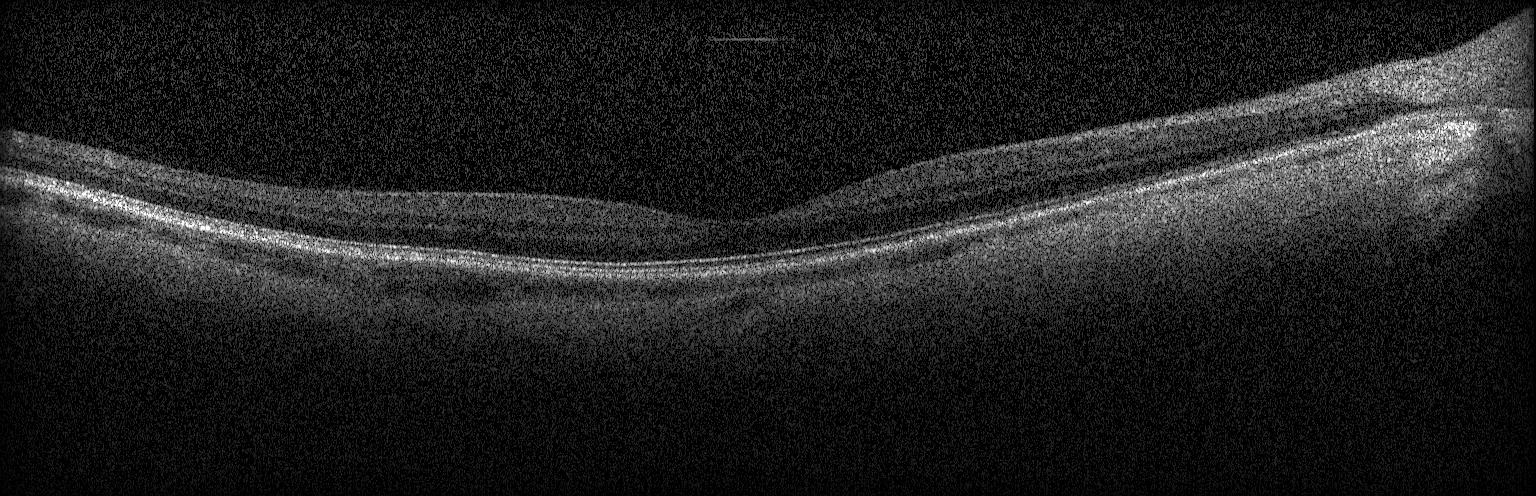

Diagnosis: no choroidal neovascularization, no diabetic macular edema, and no drusen.